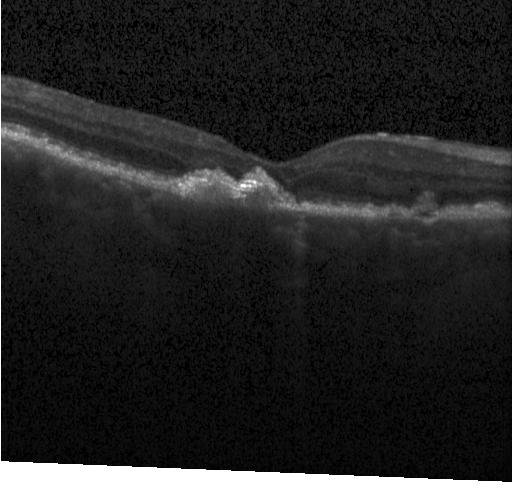 Retinal OCT cross-section.
The scan shows a choroidal neovascular membrane.